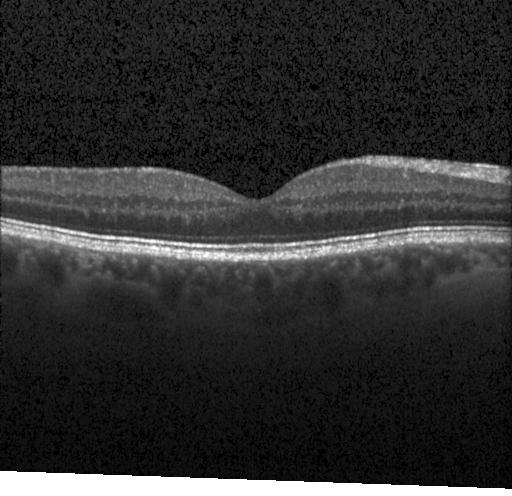 Diagnosis: no evidence of CNV, DME, or drusen.